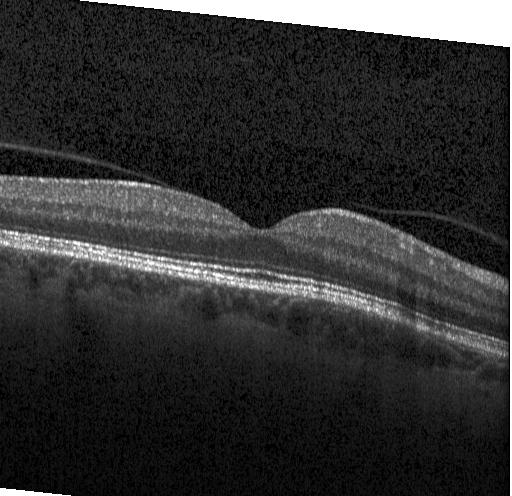 Fovea-centered. SD-OCT. Optical coherence tomography B-scan. OCT finding: no CNV, DME, or drusen.